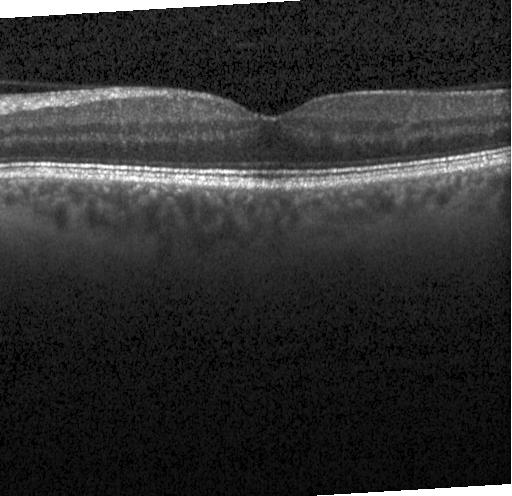 SD-OCT · centered on the fovea · OCT line scan
Impression: no choroidal neovascularization, diabetic macular edema, or drusen.